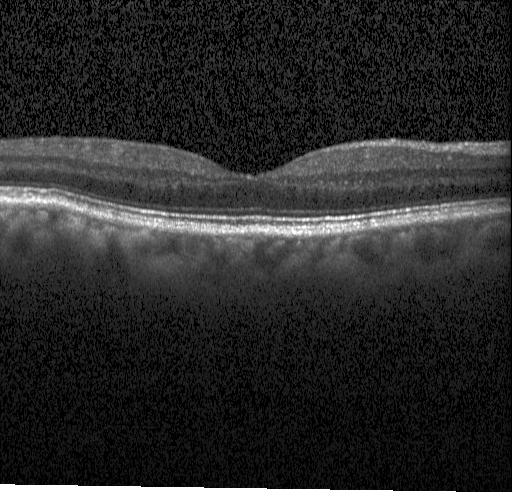
Macular OCT: neither CNV, DME, nor drusen.